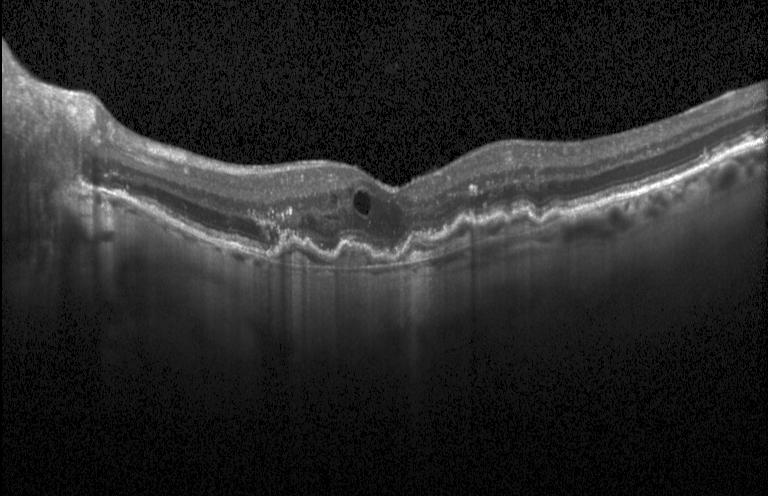 OCT B-scan
This B-scan demonstrates a choroidal neovascular membrane.